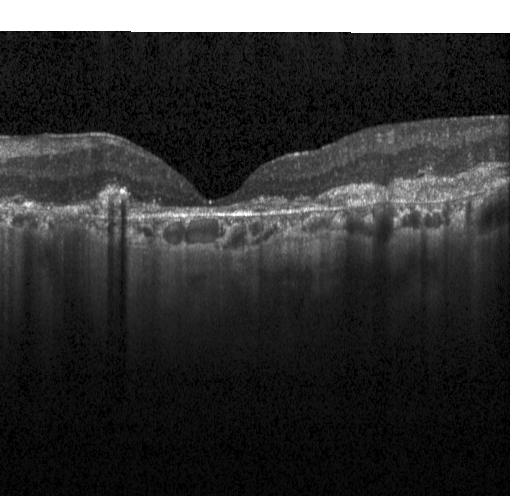

Retinal OCT cross-section · SD-OCT.
Impression: CNV.